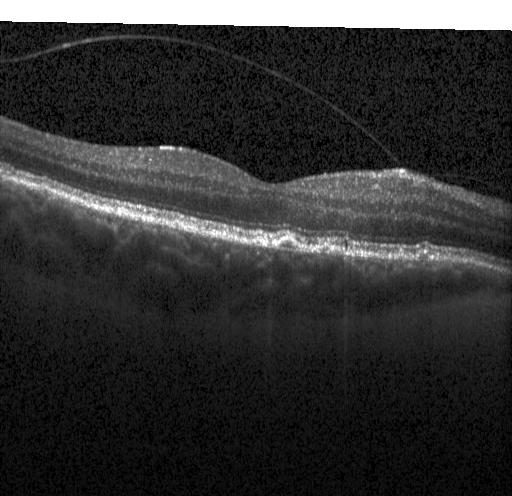 Retinal OCT cross-section — The scan shows sub-RPE drusenoid deposits.